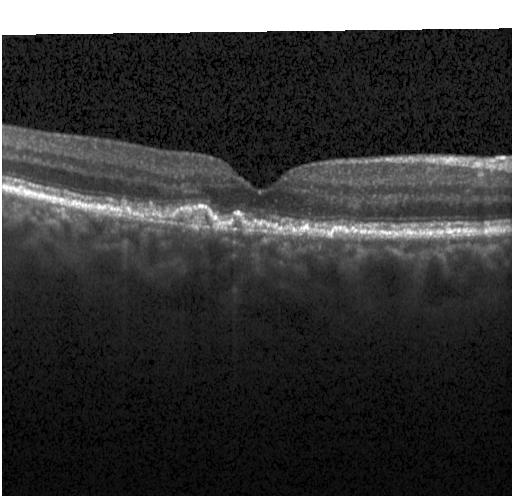 CNV.